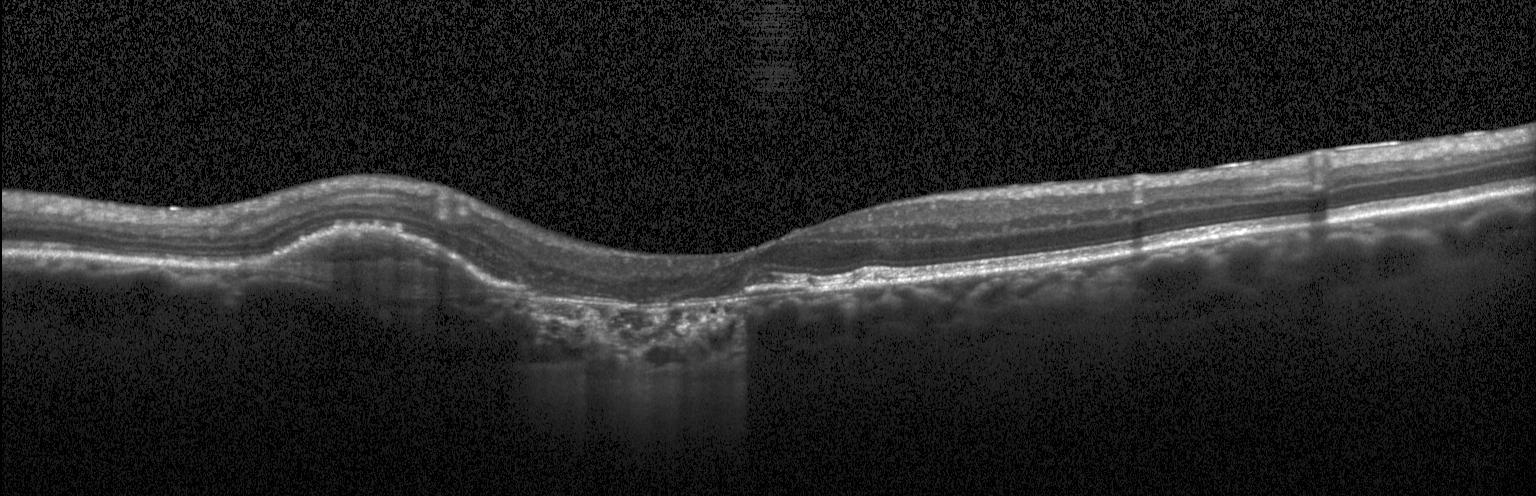
Optical coherence tomography scan, through the macula.
Dx: a choroidal neovascular membrane.